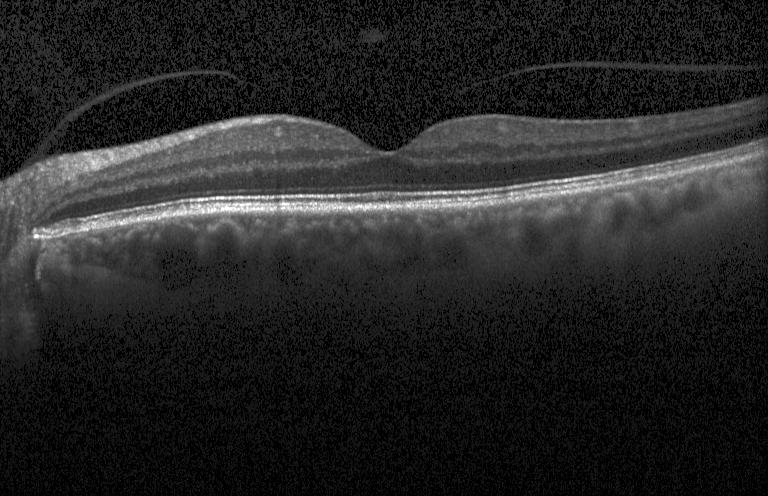
Instrument: Heidelberg Spectralis · SD-OCT · optical coherence tomography B-scan
Diagnosis: no choroidal neovascularization, diabetic macular edema, or drusen.